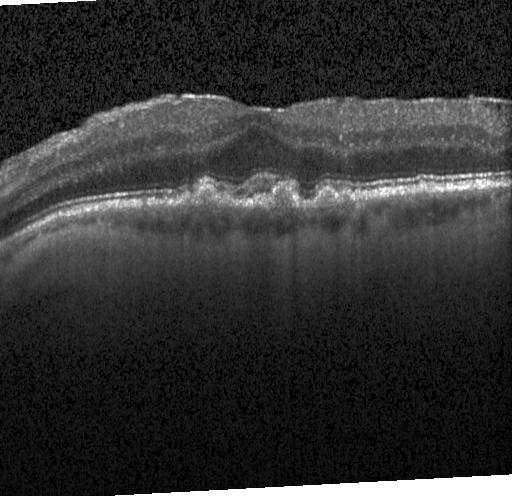 Spectral-domain OCT B-scan: sub-RPE drusenoid deposits.